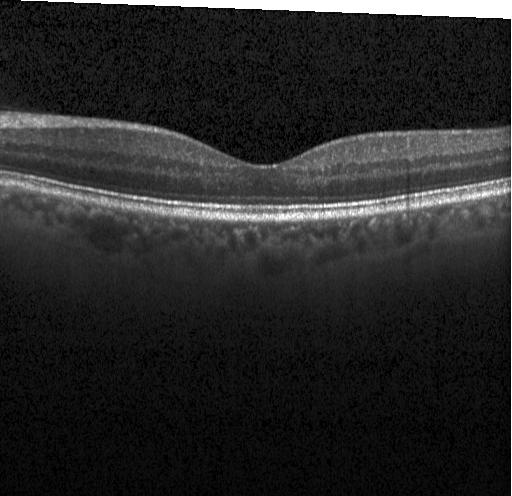

OCT finding: no choroidal neovascularization, no diabetic macular edema, and no drusen.